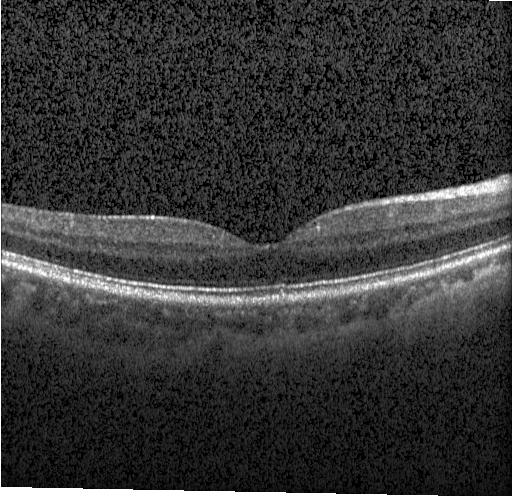

SD-OCT · instrument: Heidelberg Spectralis · optical coherence tomography B-scan · horizontal scan through the fovea — Finding: neither CNV, DME, nor drusen.